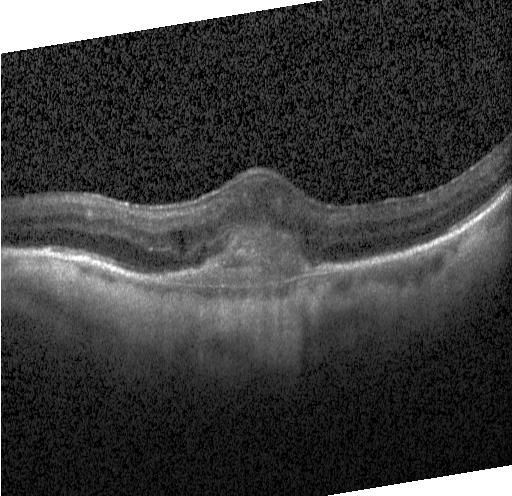
Instrument: Heidelberg Spectralis, OCT B-scan, macular scan
OCT finding: CNV.